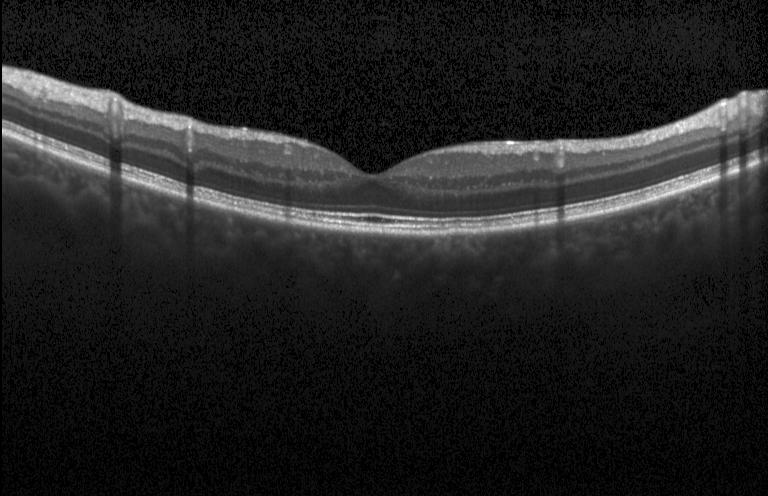 OCT scan showing no choroidal neovascularization, diabetic macular edema, or drusen.